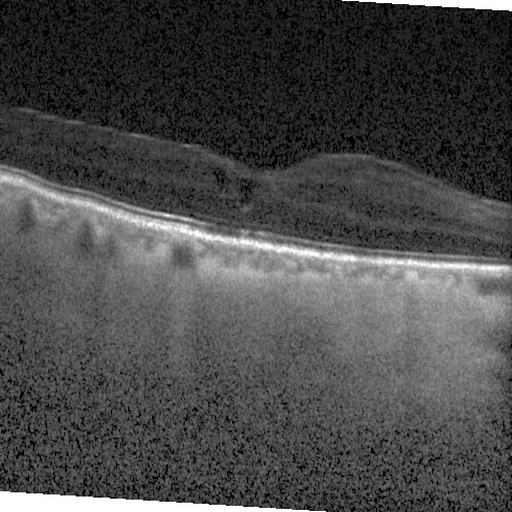

This B-scan demonstrates diabetic macular edema (DME).